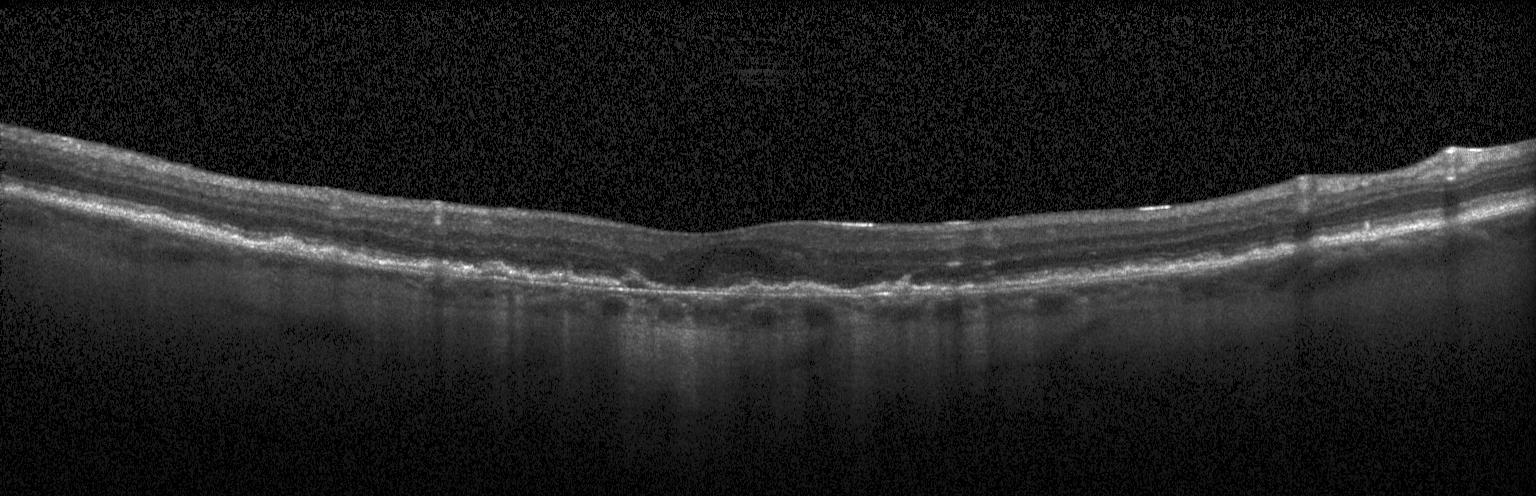

Finding: a choroidal neovascular membrane.